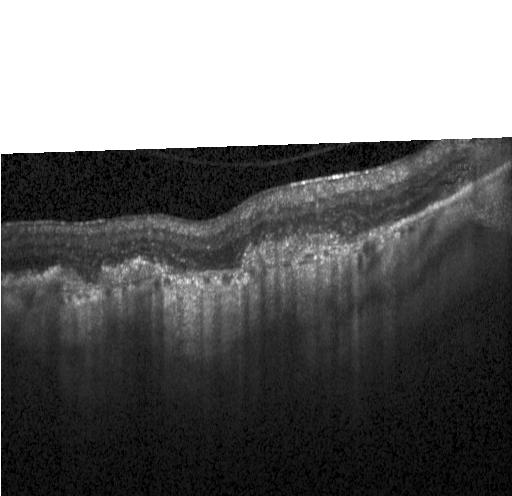
Dx: a choroidal neovascular membrane.